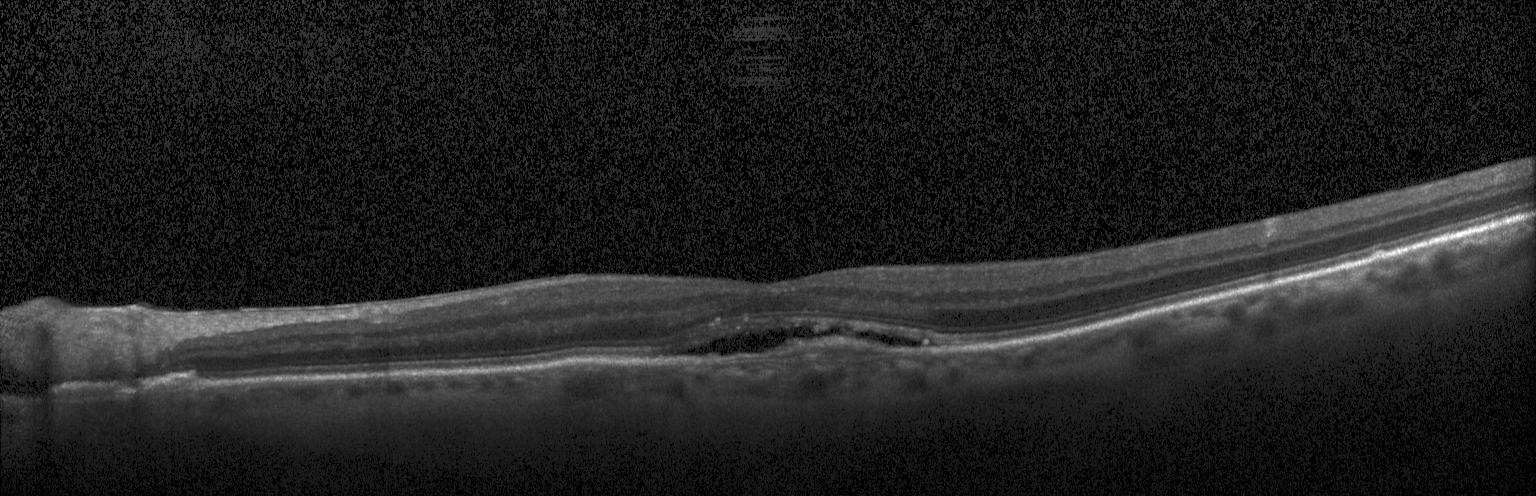 Macular OCT: a choroidal neovascular membrane.